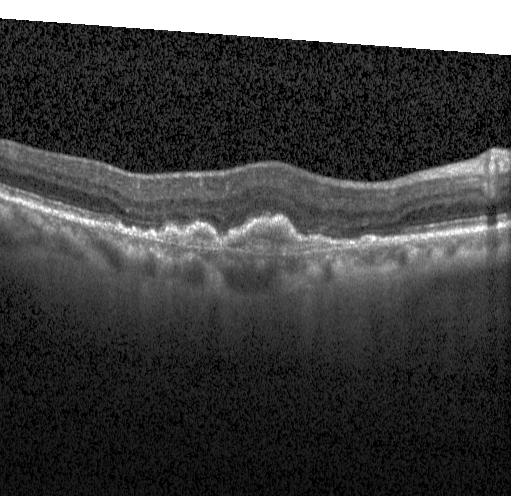 This B-scan demonstrates a choroidal neovascular membrane.